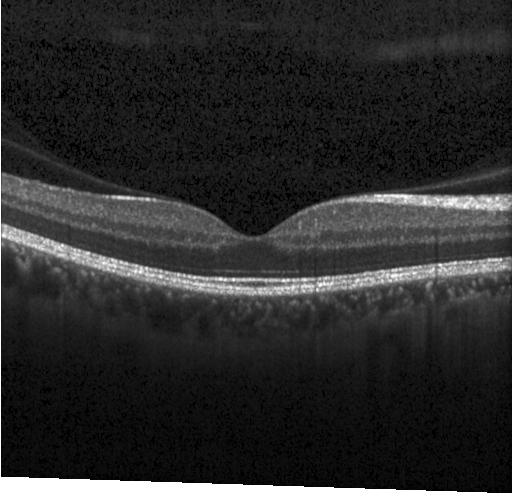

Impression: no evidence of choroidal neovascularization, diabetic macular edema, or drusen.